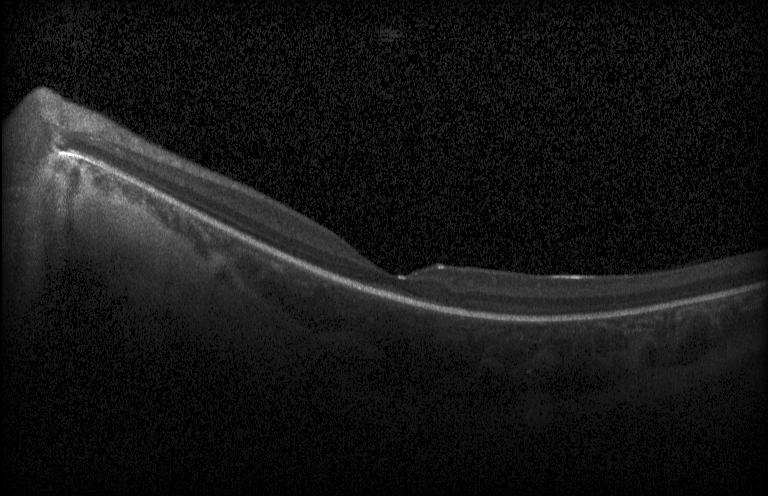
Spectral-domain OCT · Heidelberg Spectralis OCT system · OCT line scan · macular scan. Assessment: no evidence of choroidal neovascularization, diabetic macular edema, or drusen.